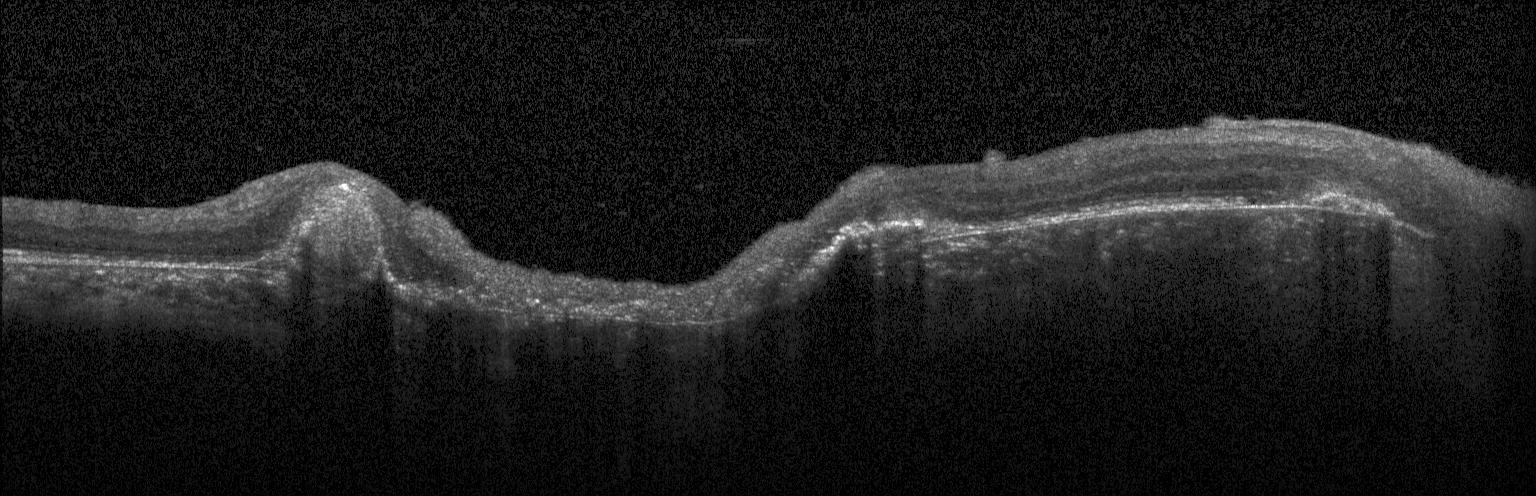

Impression: CNV.